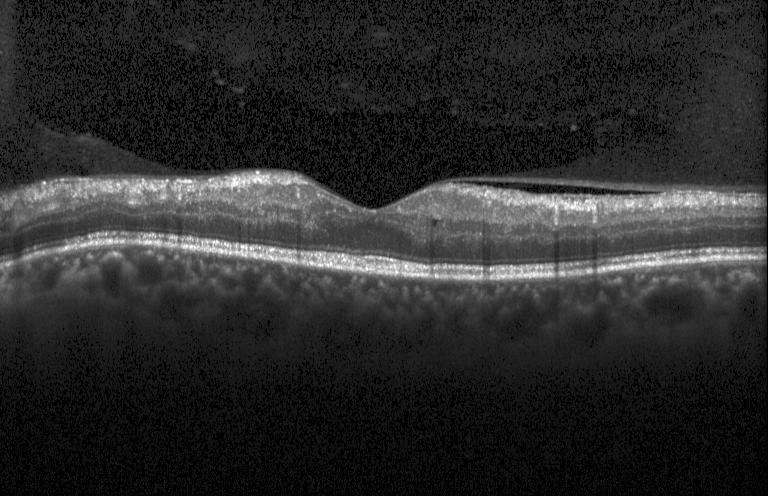 OCT B-scan showing diabetic macular edema (DME).